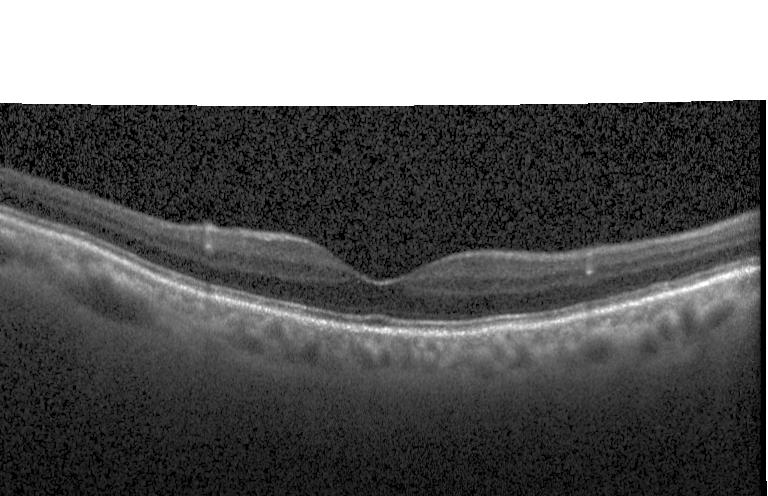 Assessment: neither CNV, DME, nor drusen.